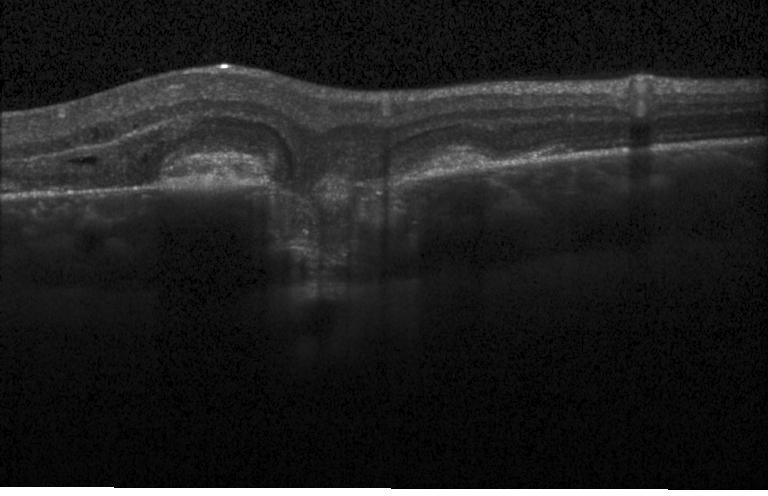

Through the macula, SD-OCT, OCT B-scan, Heidelberg Spectralis OCT system
A choroidal neovascular membrane.